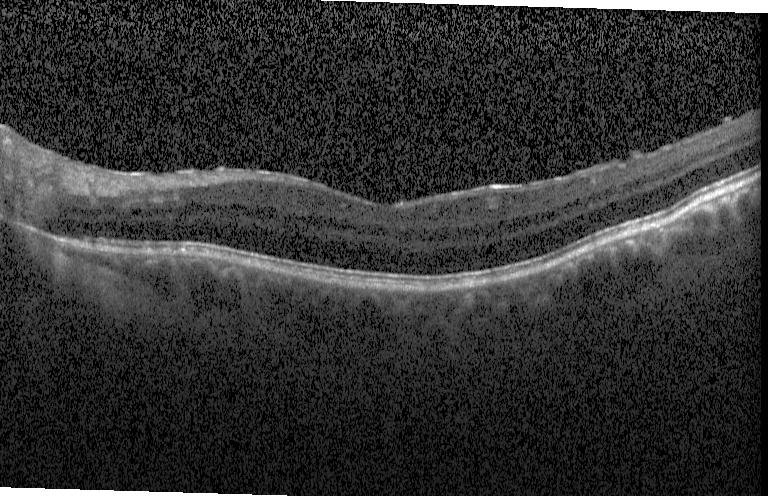
Macular OCT demonstrating no evidence of choroidal neovascularization, diabetic macular edema, or drusen.